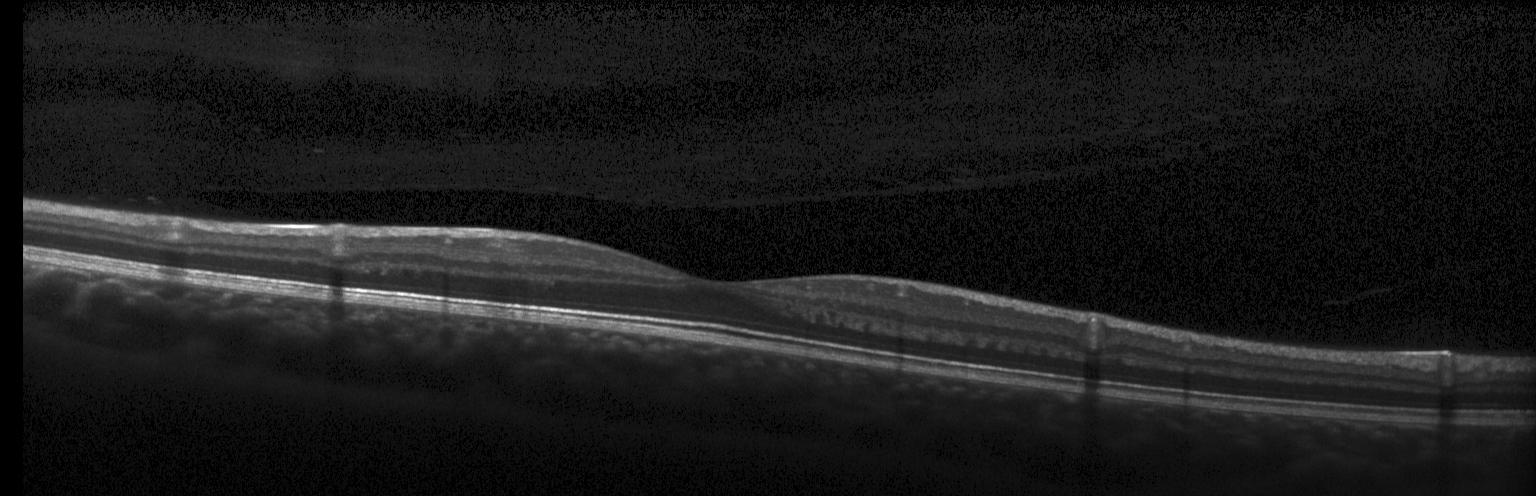 This B-scan demonstrates no choroidal neovascularization, no diabetic macular edema, and no drusen.